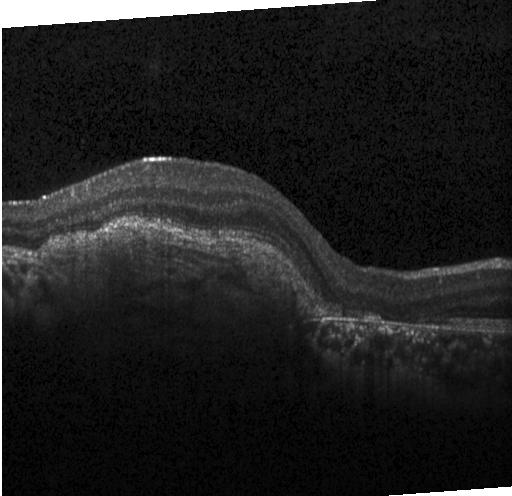
OCT scan showing a choroidal neovascular membrane.